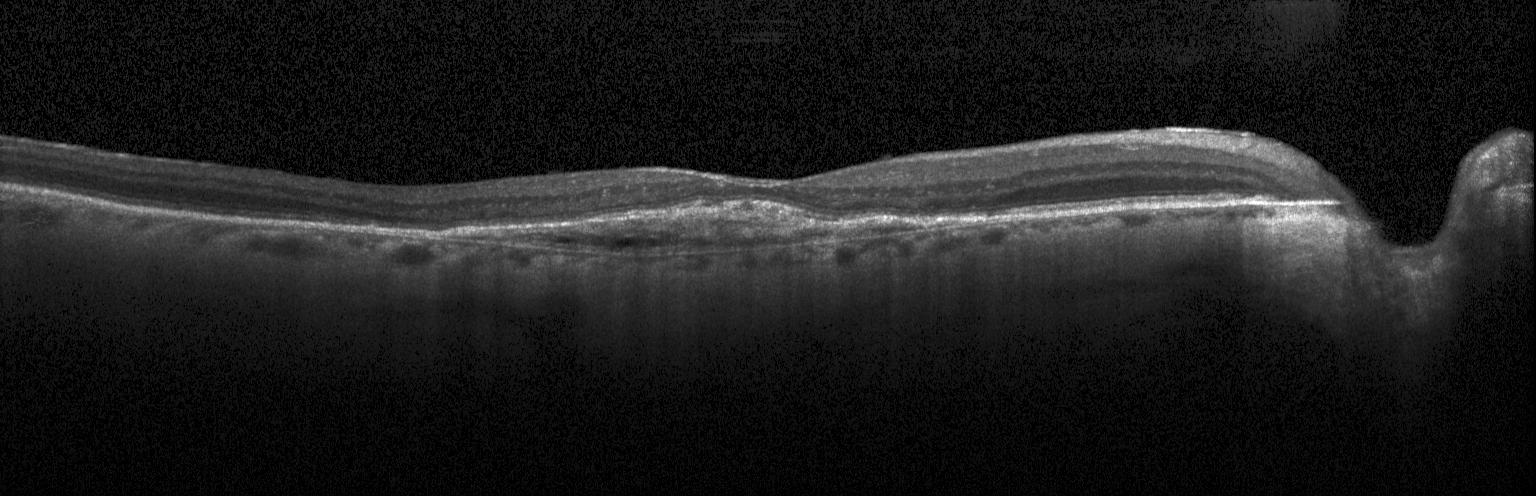 Retinal OCT cross-section
Impression: CNV.